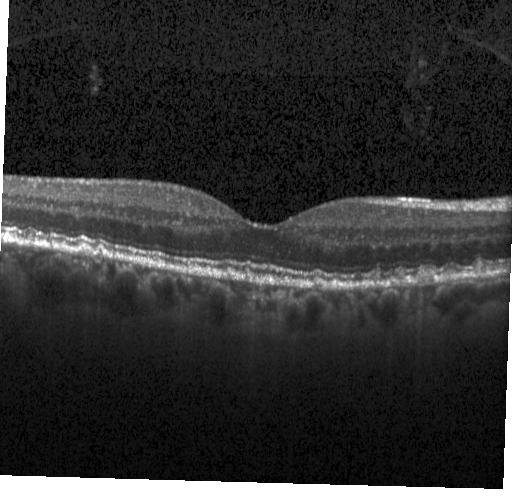 Retinal OCT B-scan. Fovea-centered.
Impression: drusen.